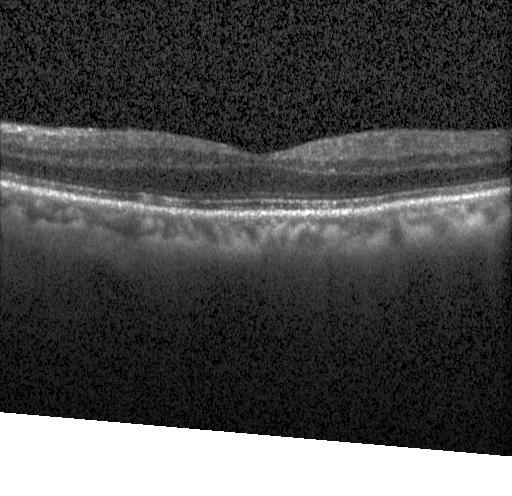 Horizontal scan through the fovea. Heidelberg Spectralis. Spectral-domain OCT. Retinal OCT B-scan — Finding: no choroidal neovascularization, diabetic macular edema, or drusen.